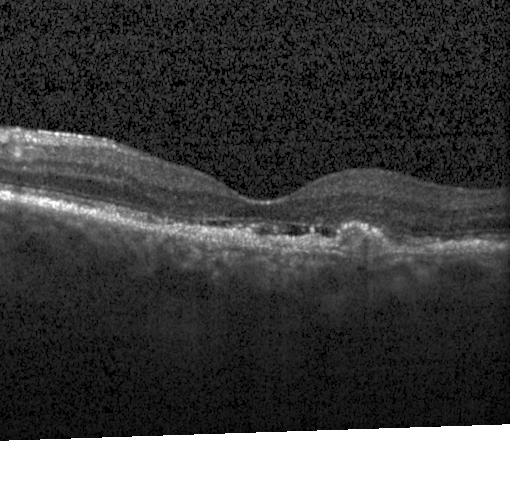

Dx: a choroidal neovascular membrane.